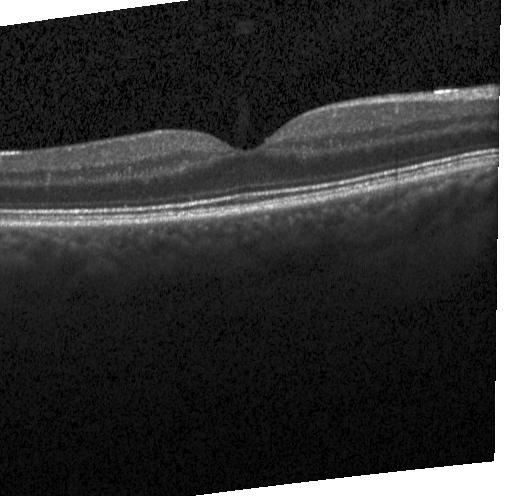

Instrument: Heidelberg Spectralis · retinal OCT cross-section.
Impression: no evidence of choroidal neovascularization, diabetic macular edema, or drusen.